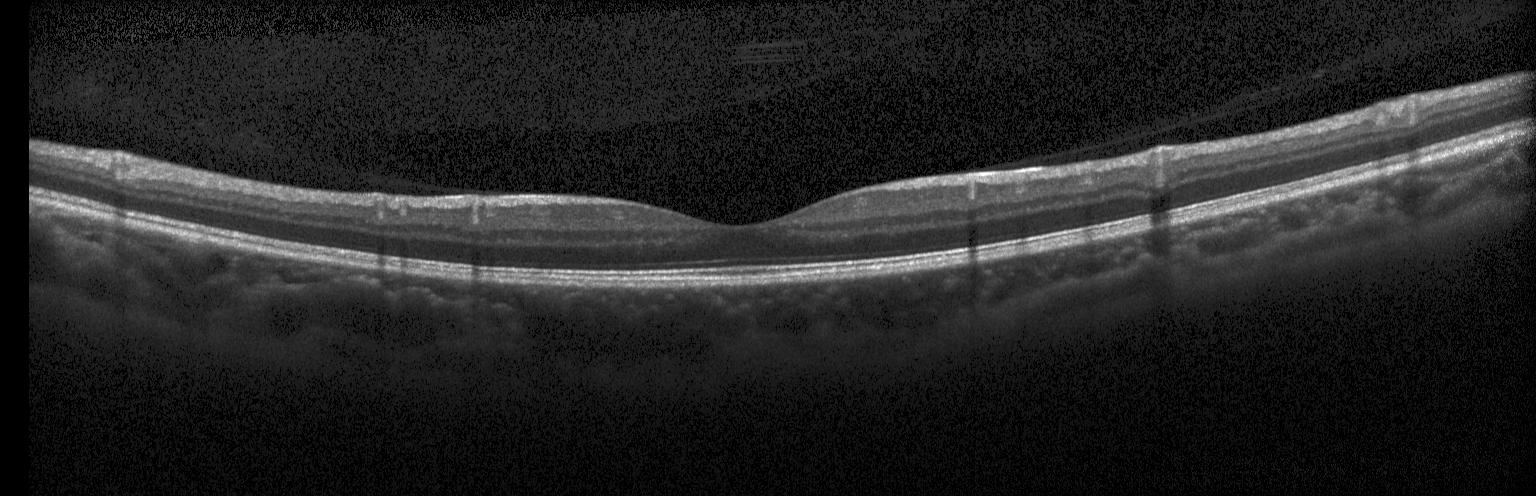 Macular OCT demonstrating no choroidal neovascularization, no diabetic macular edema, and no drusen.